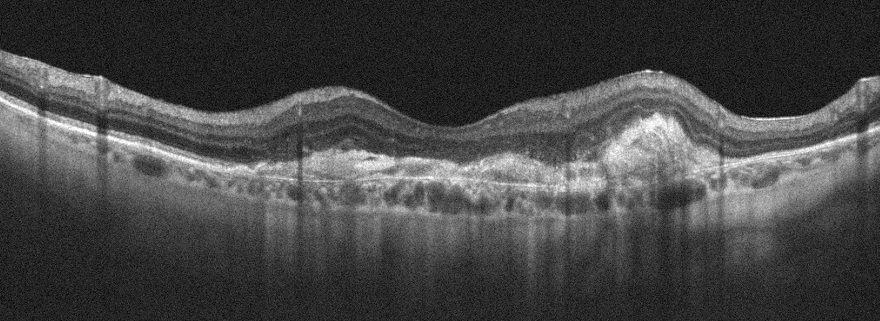

Diagnosis: age-related macular degeneration (AMD).